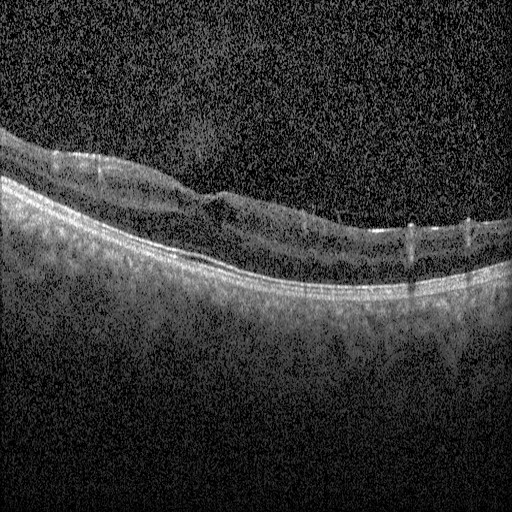 Fovea-centered · OCT B-scan · spectral-domain OCT.
Dx: diabetic macular edema.